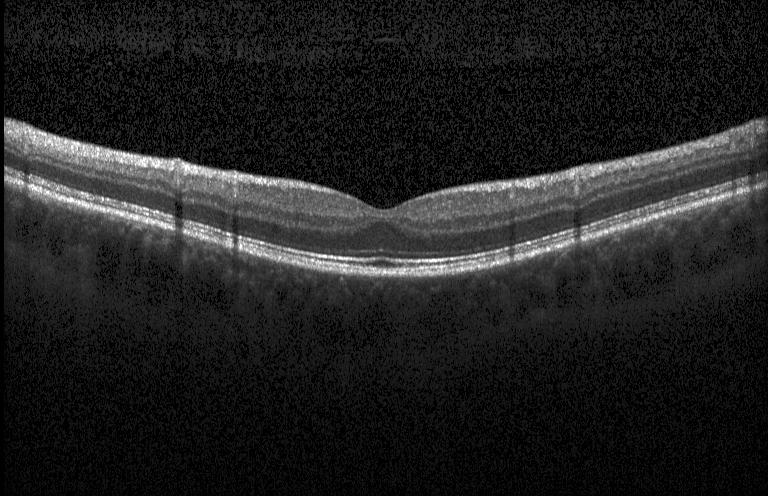 Impression: no CNV, DME, or drusen.